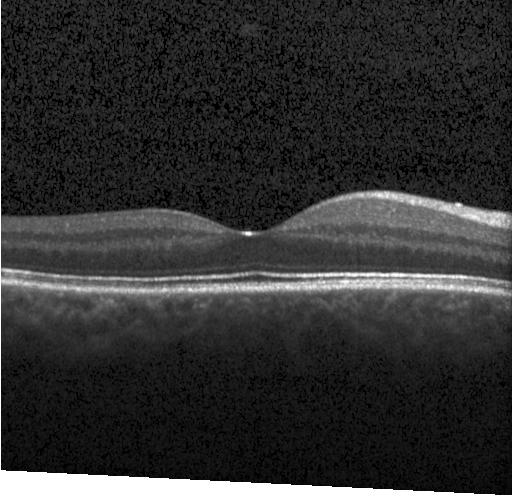
Optical coherence tomography scan.
Macular OCT: no CNV, no DME, and no drusen.